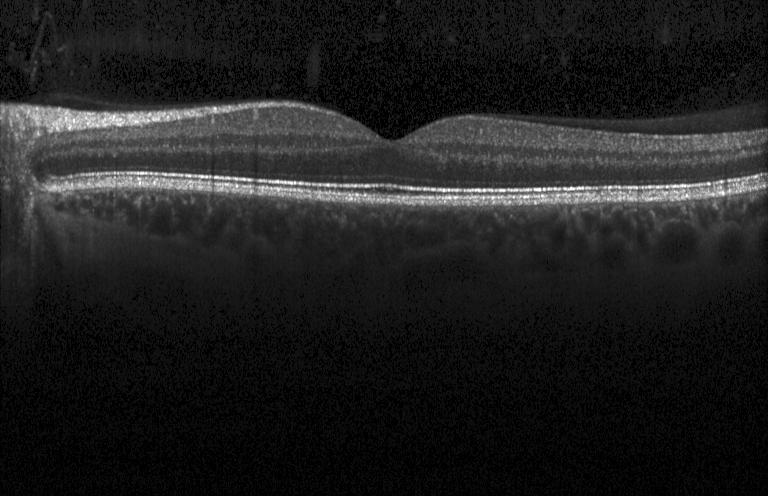
OCT line scan · through the macula — Finding: no choroidal neovascularization, diabetic macular edema, or drusen.